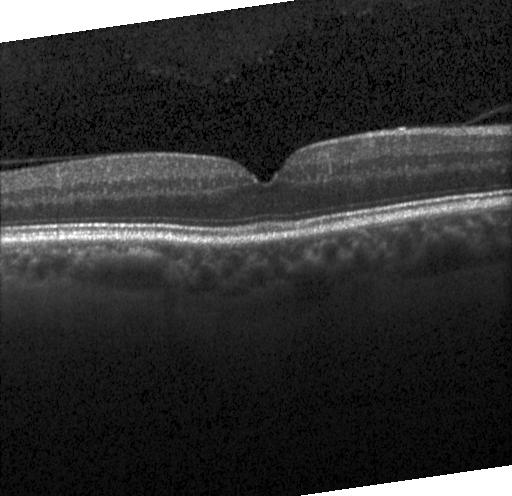 Heidelberg Spectralis OCT system; through the macula; retinal OCT cross-section; SD-OCT. OCT finding: no choroidal neovascularization, diabetic macular edema, or drusen.